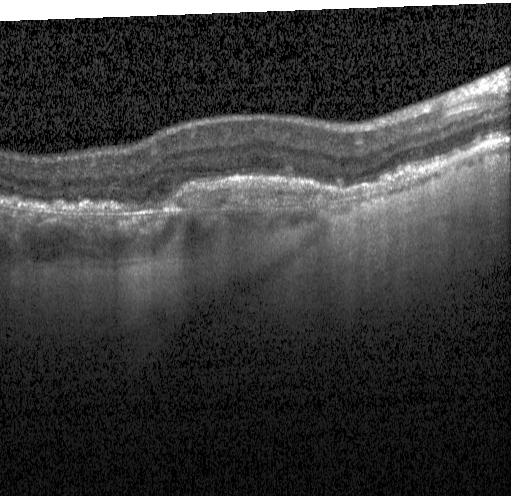
Horizontal scan through the fovea, retinal OCT B-scan, SD-OCT
This B-scan demonstrates a choroidal neovascular membrane.